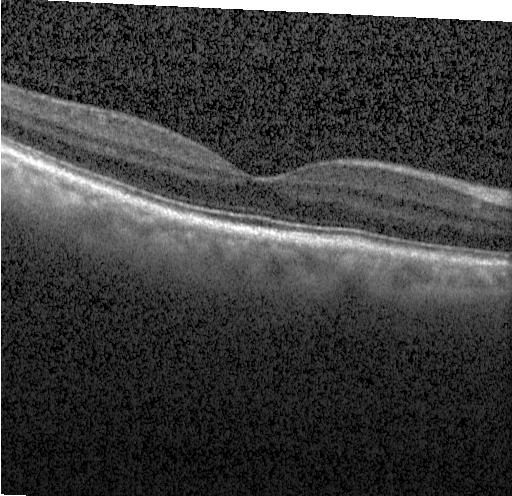

Instrument: Heidelberg Spectralis · SD-OCT · optical coherence tomography B-scan. Finding: no choroidal neovascularization, no diabetic macular edema, and no drusen.